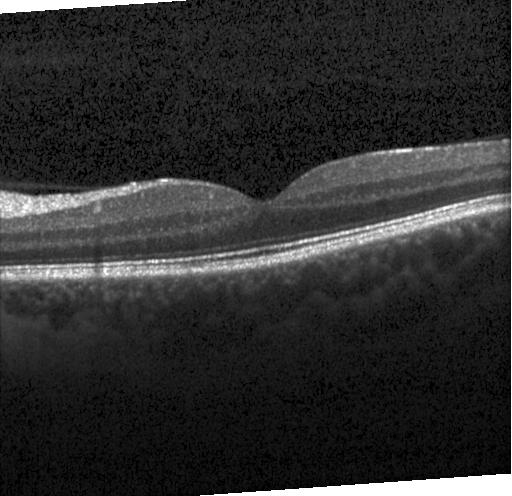
SD-OCT; OCT B-scan; centered on the fovea; Heidelberg Spectralis OCT system
Diagnosis: neither choroidal neovascularization, diabetic macular edema, nor drusen.